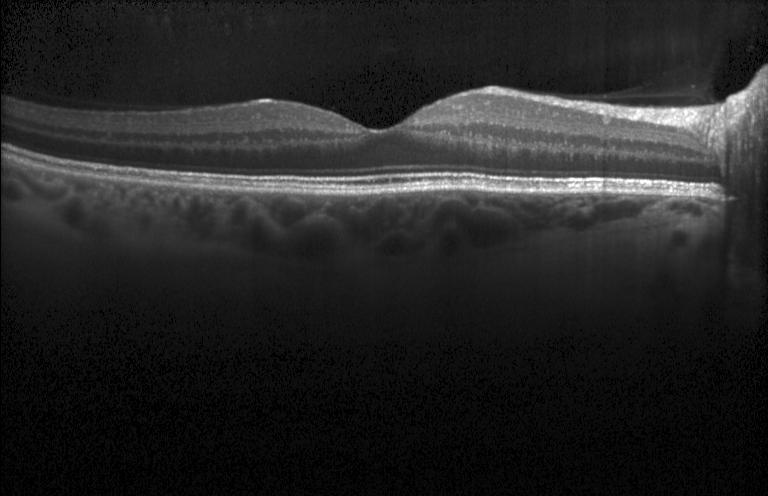 OCT B-scan; spectral-domain optical coherence tomography; macular scan; acquired on a Heidelberg Spectralis
Diagnosis: no evidence of choroidal neovascularization, diabetic macular edema, or drusen.